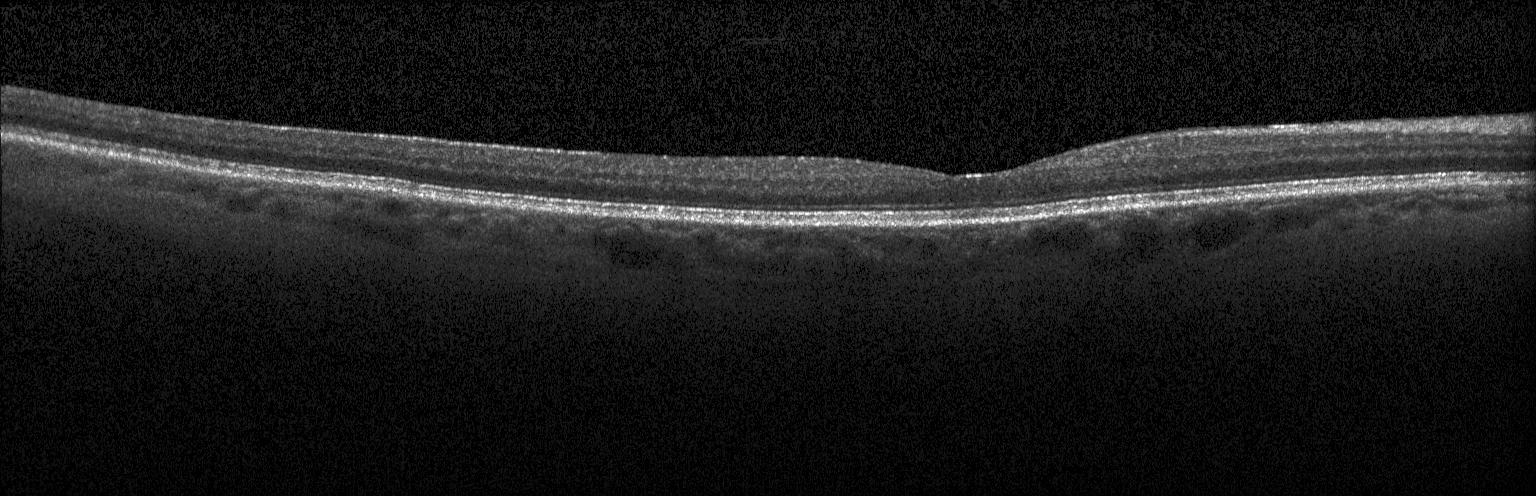

Optical coherence tomography B-scan · spectral-domain OCT · fovea-centered · Heidelberg Spectralis
Diagnosis: neither choroidal neovascularization, diabetic macular edema, nor drusen.